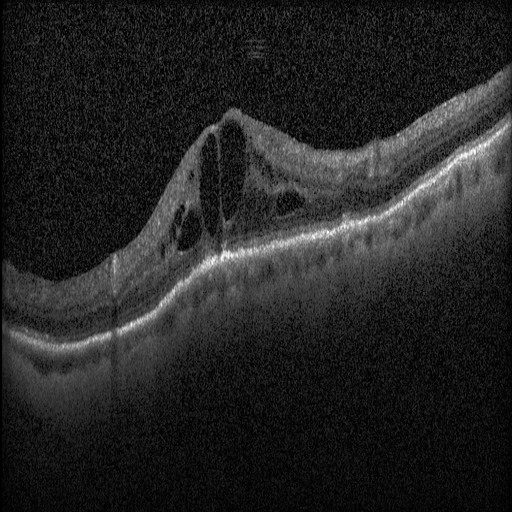
Assessment: diabetic macular edema (DME).